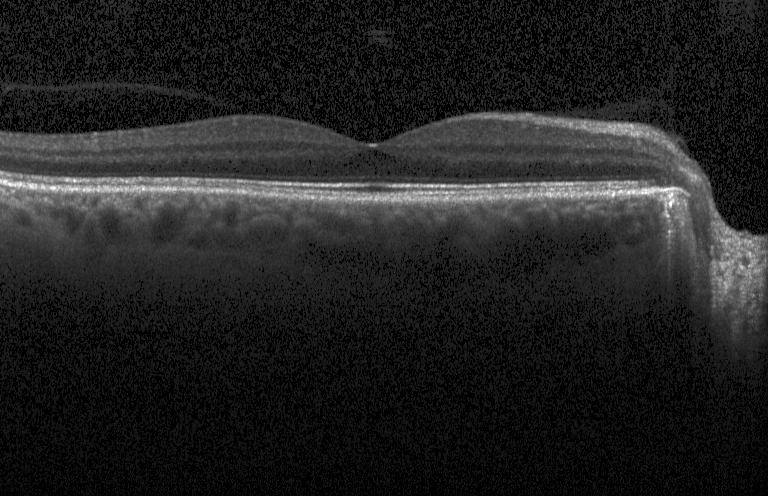

No choroidal neovascularization, diabetic macular edema, or drusen.